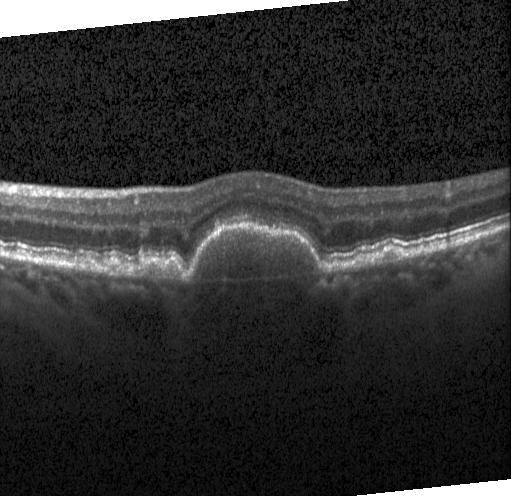 Retinal OCT B-scan
OCT finding: a choroidal neovascular membrane.